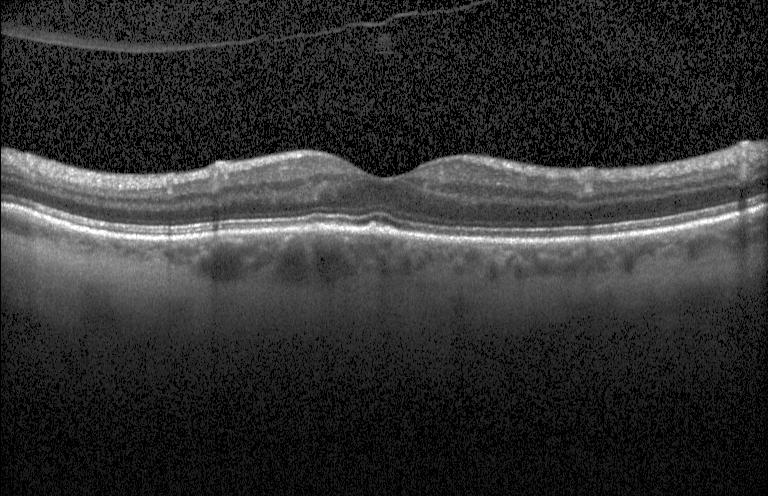
Macular OCT demonstrating sub-RPE drusenoid deposits.